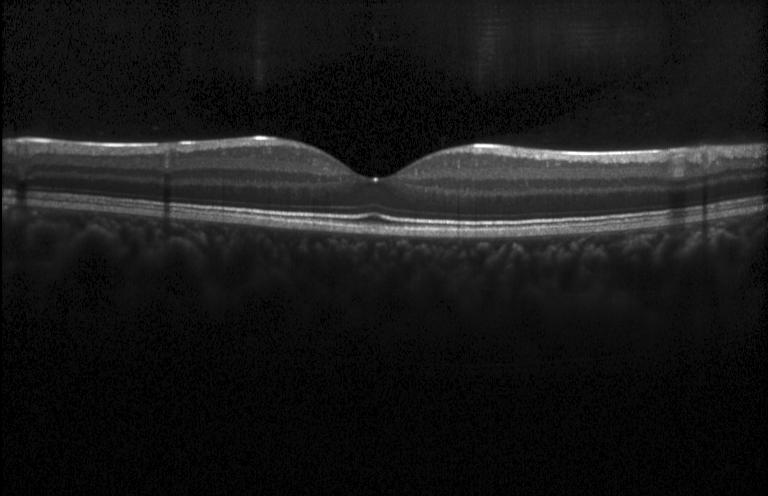

Retinal OCT B-scan; acquired on a Heidelberg Spectralis; horizontal scan through the fovea; SD-OCT. The scan shows no CNV, no DME, and no drusen.